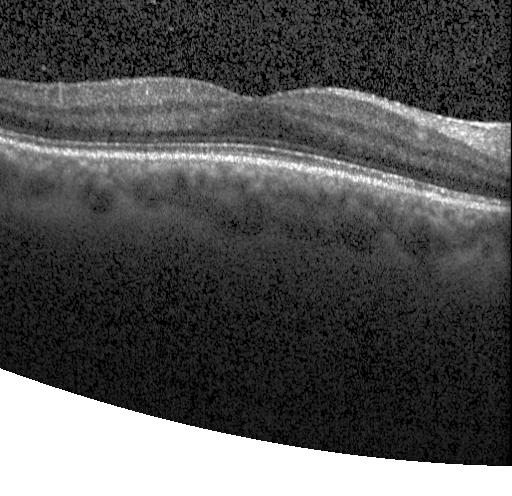

Retinal OCT cross-section
No CNV, no DME, and no drusen.